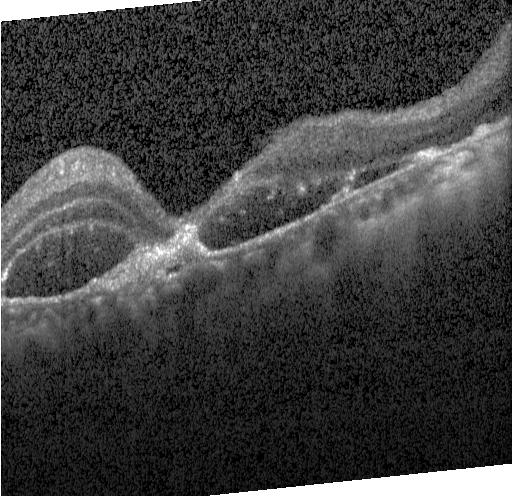
CNV.